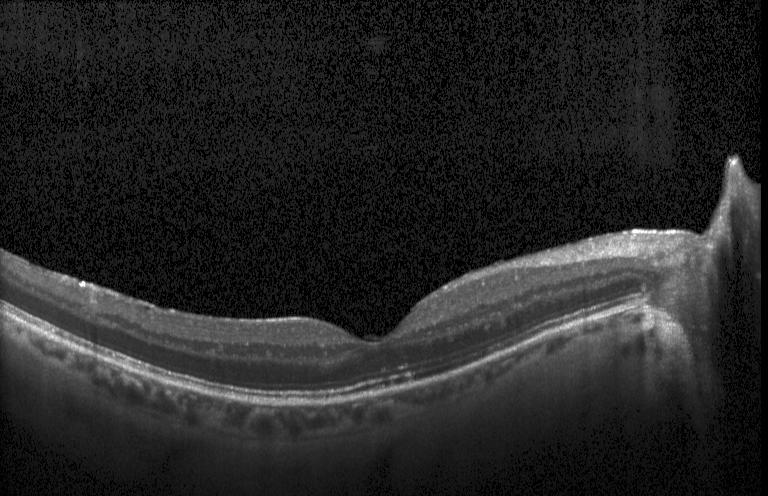 Optical coherence tomography scan — Dx: no CNV, DME, or drusen.